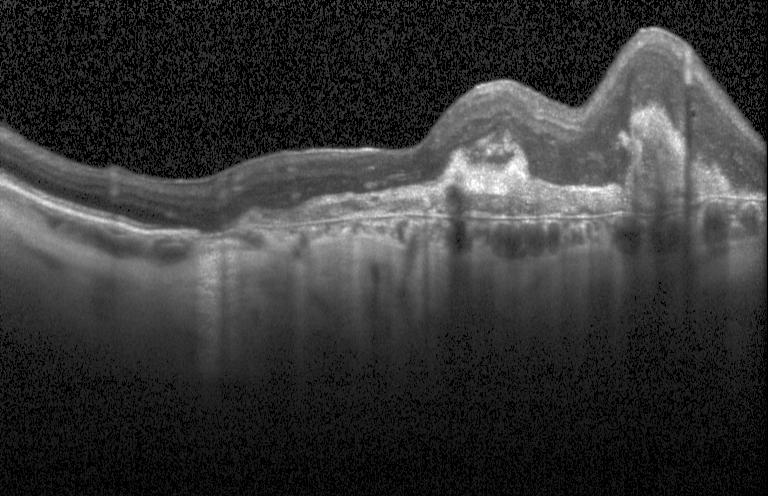

Diagnosis: a choroidal neovascular membrane.